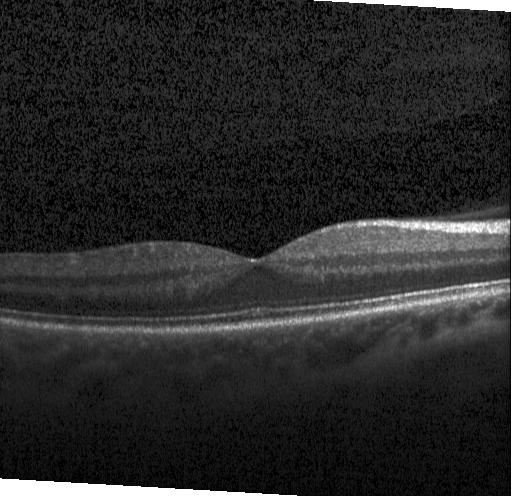 The scan shows neither choroidal neovascularization, diabetic macular edema, nor drusen.